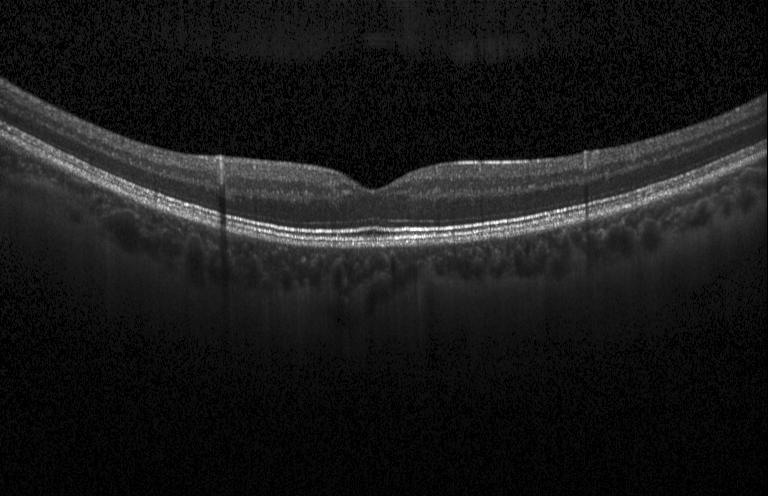 OCT scan showing neither CNV, DME, nor drusen.